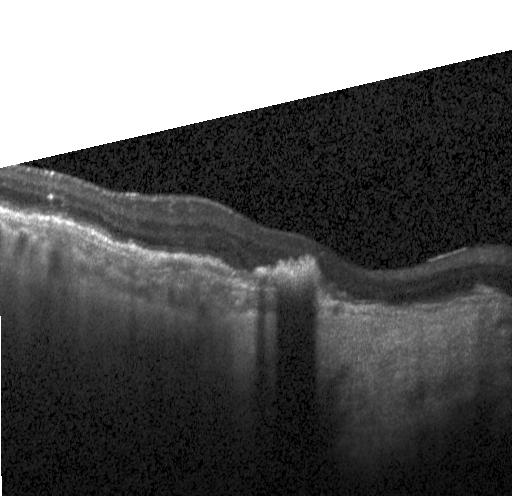

Horizontal scan through the fovea · optical coherence tomography scan · instrument: Heidelberg Spectralis
The scan shows choroidal neovascularization.